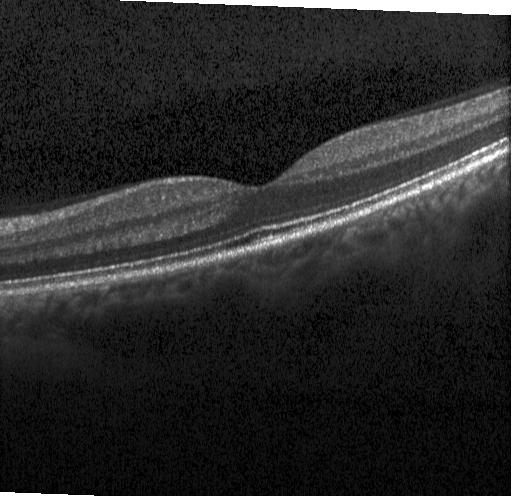 Centered on the fovea. Retinal OCT cross-section. Spectral-domain OCT. Instrument: Heidelberg Spectralis
Finding: no CNV, DME, or drusen.